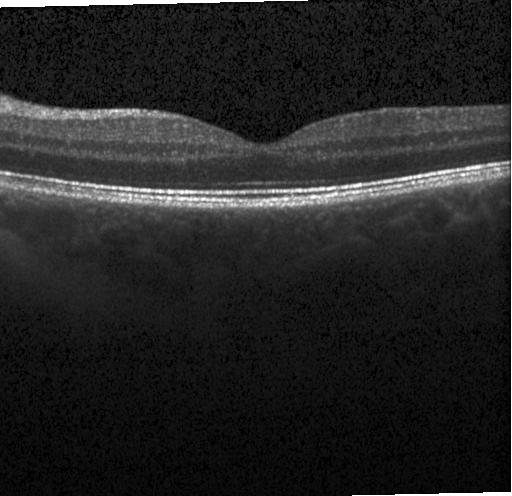

This B-scan demonstrates no choroidal neovascularization, diabetic macular edema, or drusen.